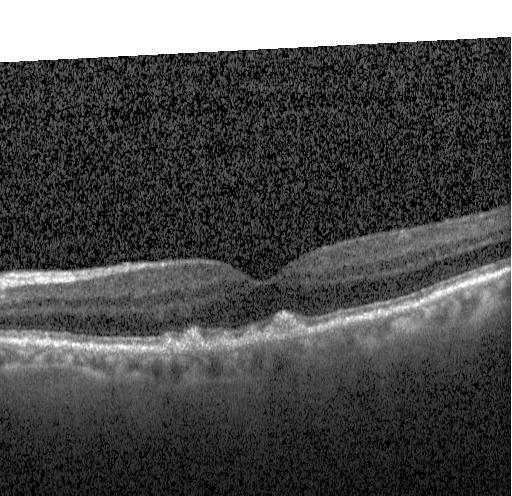 Spectral-domain OCT · retinal OCT cross-section · instrument: Heidelberg Spectralis
Diagnosis: drusen.